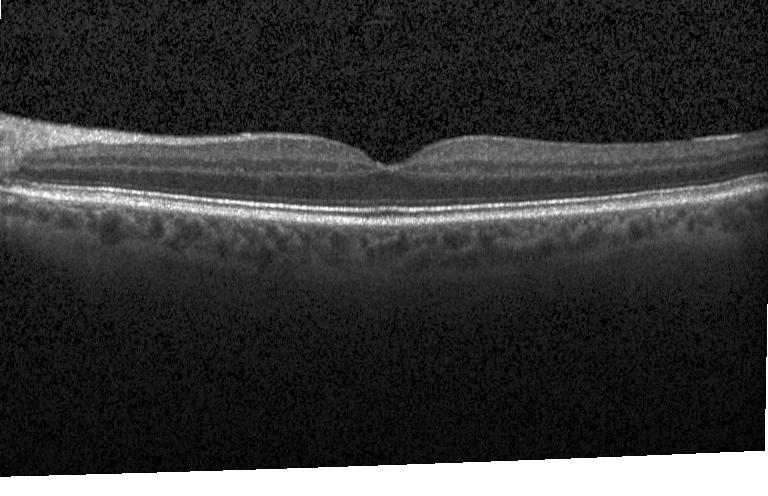

Spectral-domain OCT B-scan: no evidence of CNV, DME, or drusen.